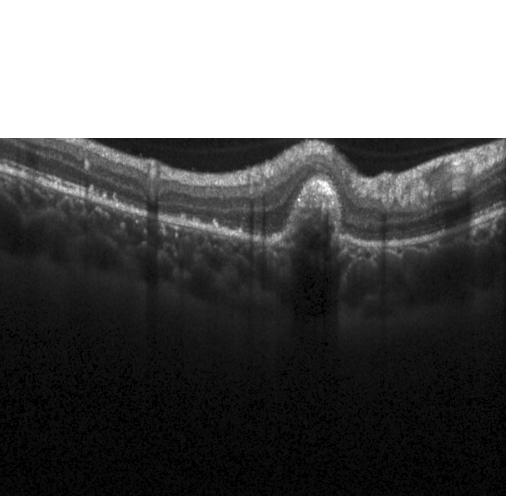 Fovea-centered · spectral-domain optical coherence tomography · optical coherence tomography B-scan
Dx: a choroidal neovascular membrane.